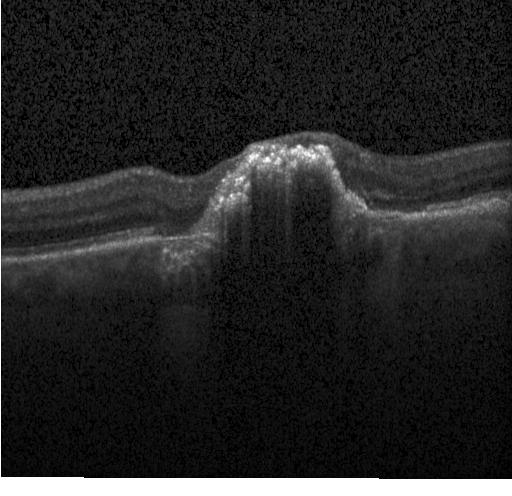 OCT finding: choroidal neovascularization.